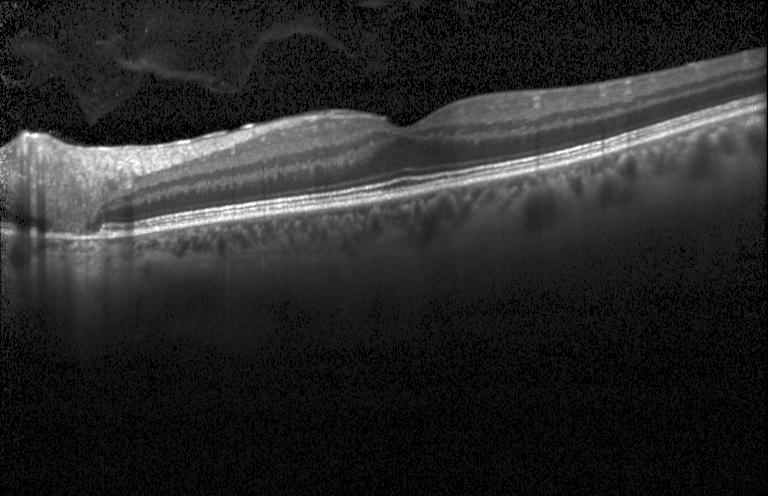

OCT finding: no evidence of choroidal neovascularization, diabetic macular edema, or drusen.